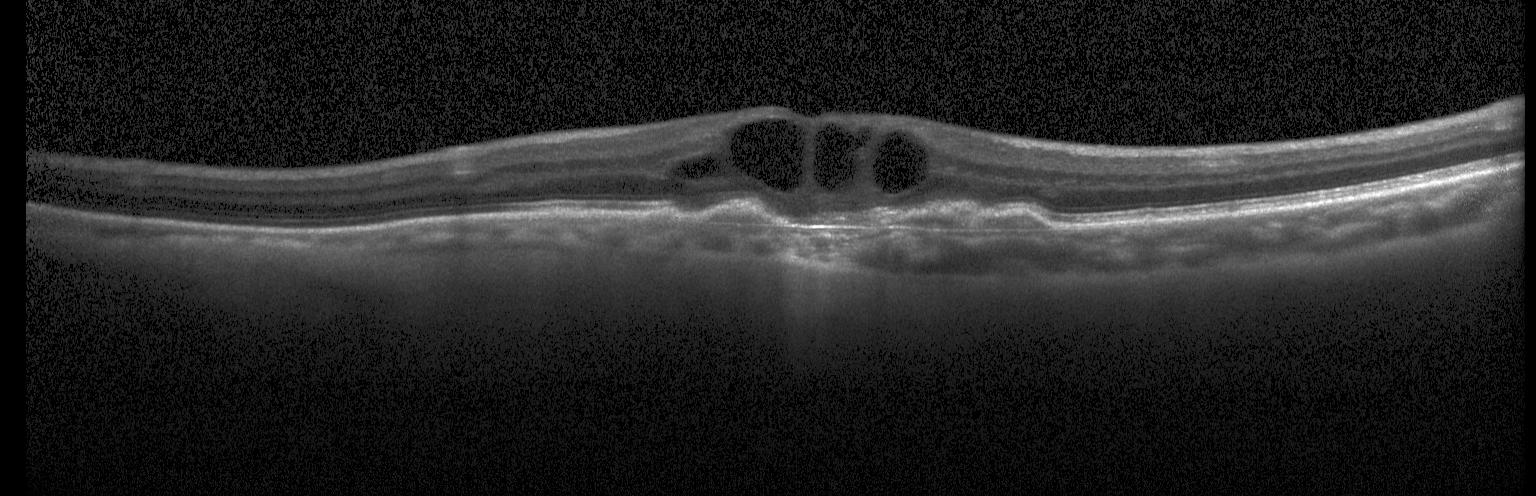

OCT finding: choroidal neovascularization (CNV).